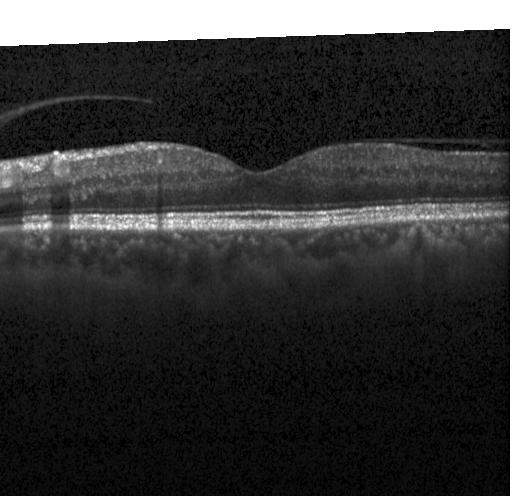
Optical coherence tomography scan · fovea-centered · SD-OCT — Diagnosis: no evidence of choroidal neovascularization, diabetic macular edema, or drusen.